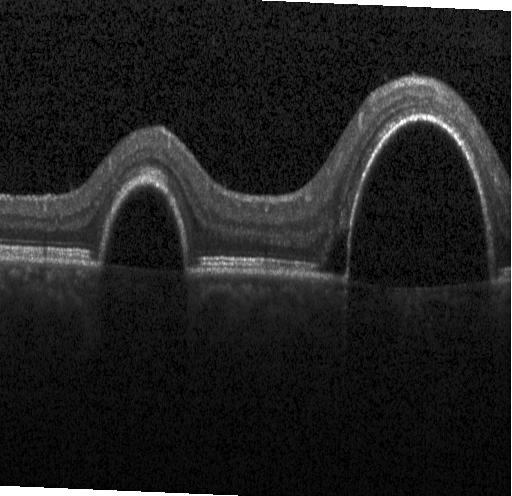

OCT B-scan
Diagnosis: a choroidal neovascular membrane.